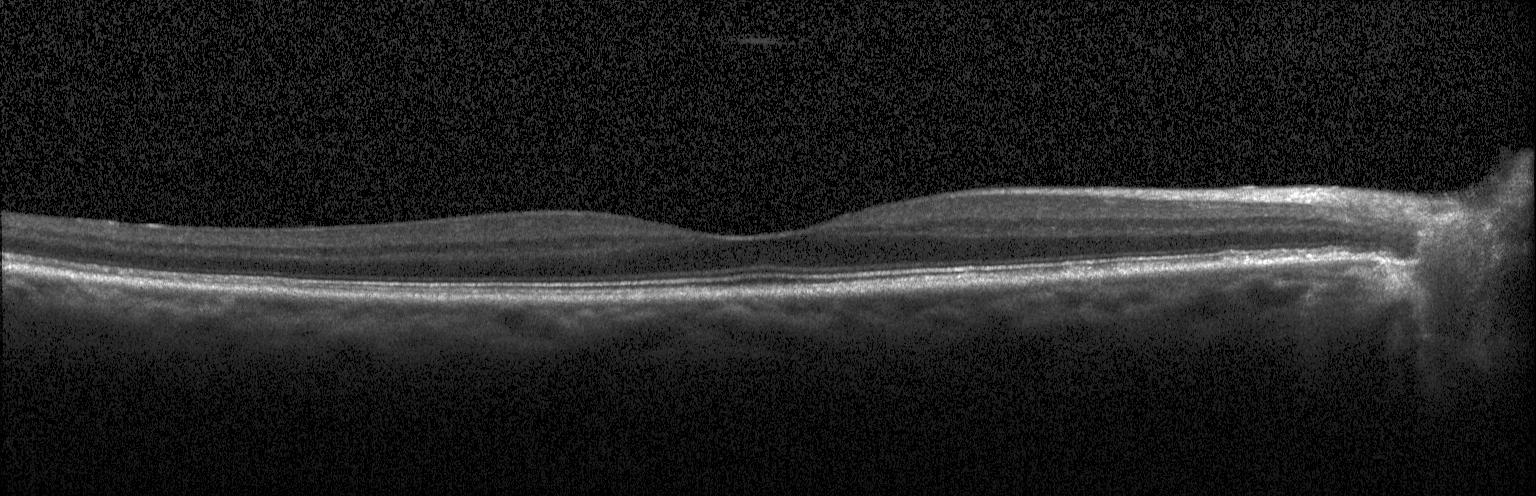

Through the macula · Heidelberg Spectralis OCT system · spectral-domain optical coherence tomography · retinal OCT cross-section
Macular OCT: no choroidal neovascularization, no diabetic macular edema, and no drusen.